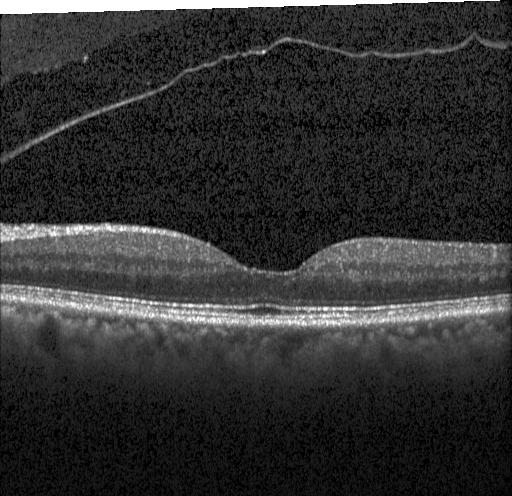
Centered on the fovea; retinal OCT cross-section. This B-scan demonstrates no CNV, no DME, and no drusen.